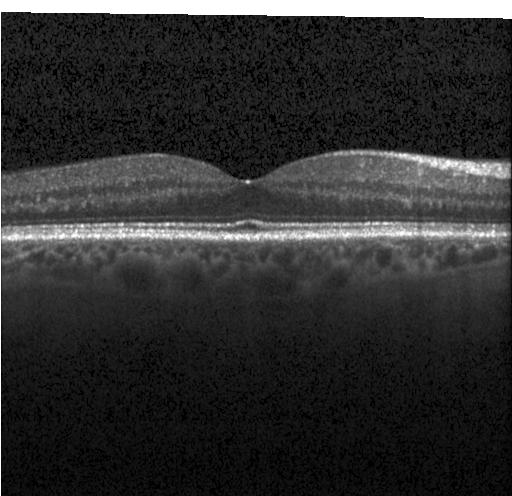

Macular OCT: no evidence of choroidal neovascularization, diabetic macular edema, or drusen.